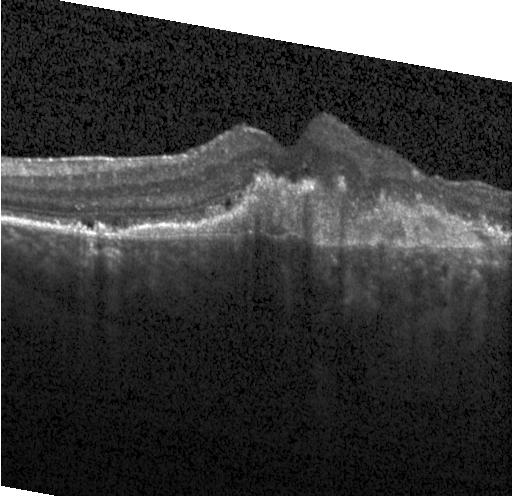

Macular OCT demonstrating choroidal neovascularization.